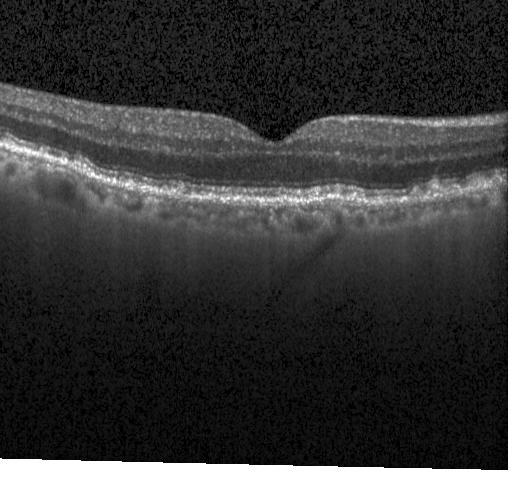 Impression: drusen.